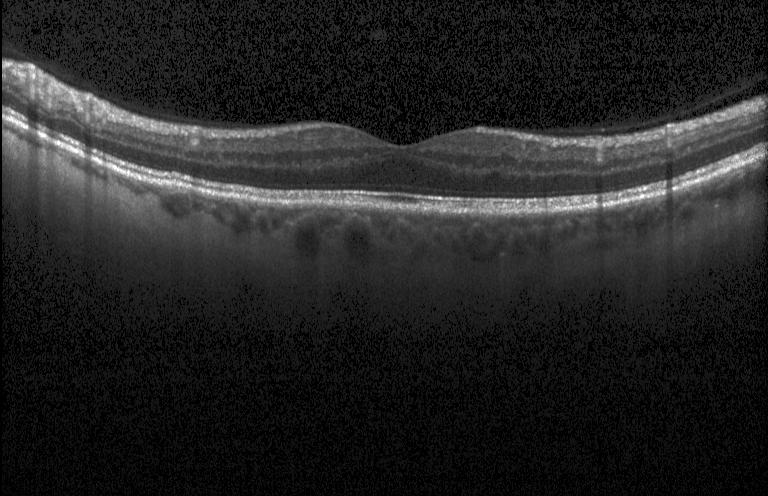 Impression: neither choroidal neovascularization, diabetic macular edema, nor drusen.